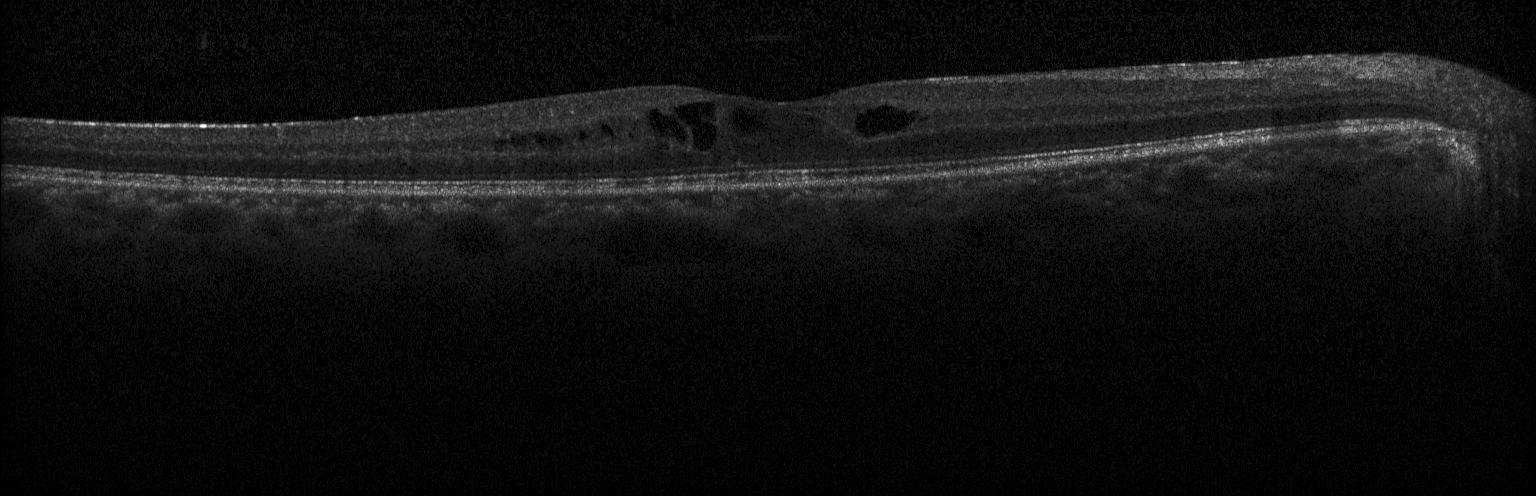
OCT line scan — Impression: DME.